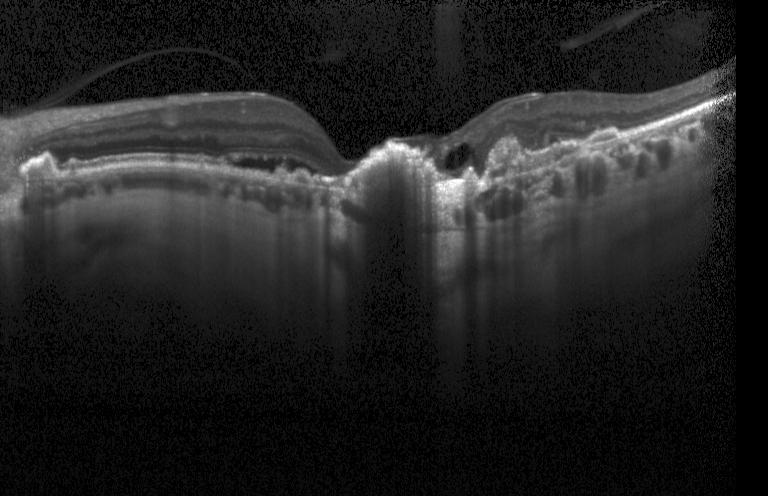 Diagnosis: a choroidal neovascular membrane.